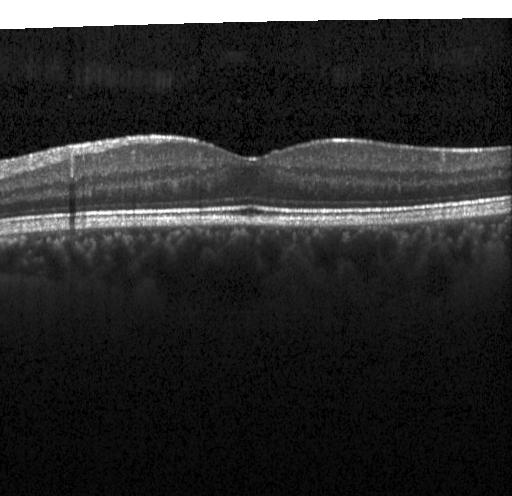
Centered on the fovea, Heidelberg Spectralis, OCT line scan, spectral-domain optical coherence tomography.
Finding: no evidence of choroidal neovascularization, diabetic macular edema, or drusen.